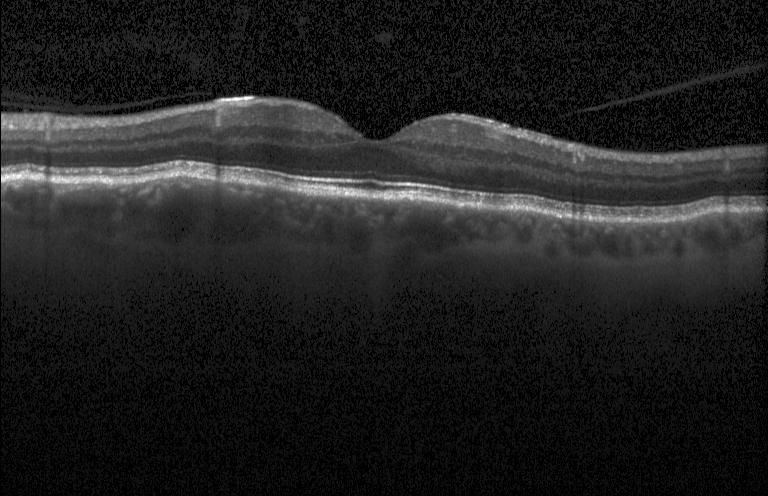

Retinal OCT B-scan · spectral-domain OCT · fovea-centered · Heidelberg Spectralis OCT system — The scan shows neither choroidal neovascularization, diabetic macular edema, nor drusen.